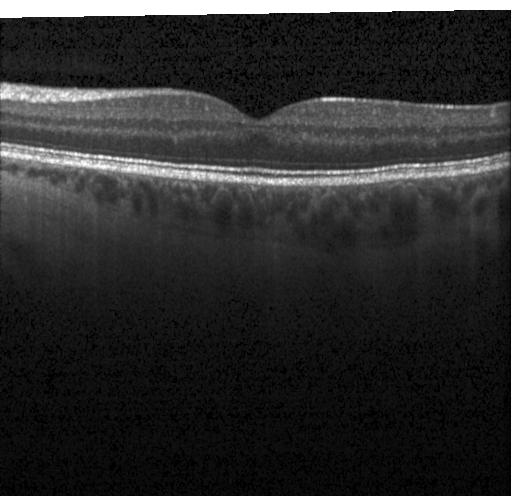
Spectral-domain OCT. Macular scan. Retinal OCT B-scan. Heidelberg Spectralis — Diagnosis: no CNV, no DME, and no drusen.